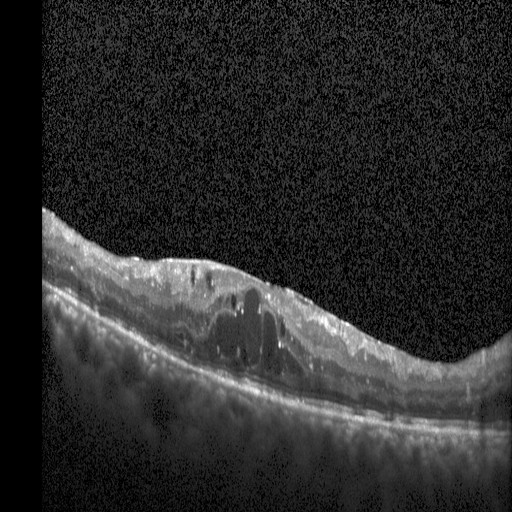

Diabetic macular edema (DME).